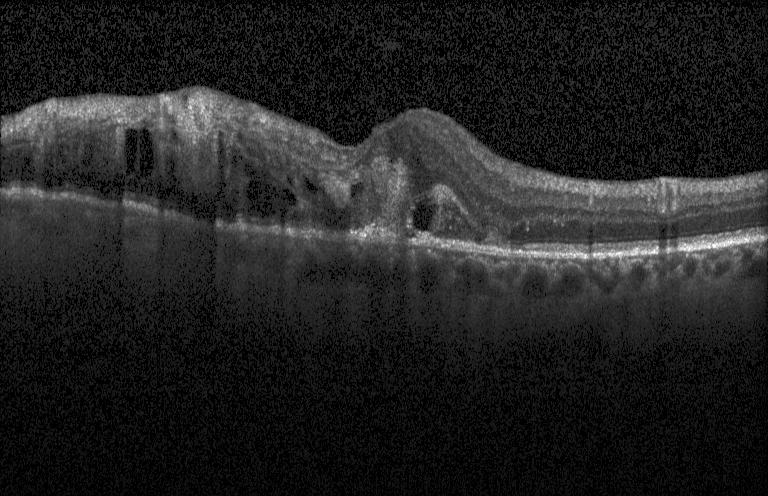

Impression: CNV.